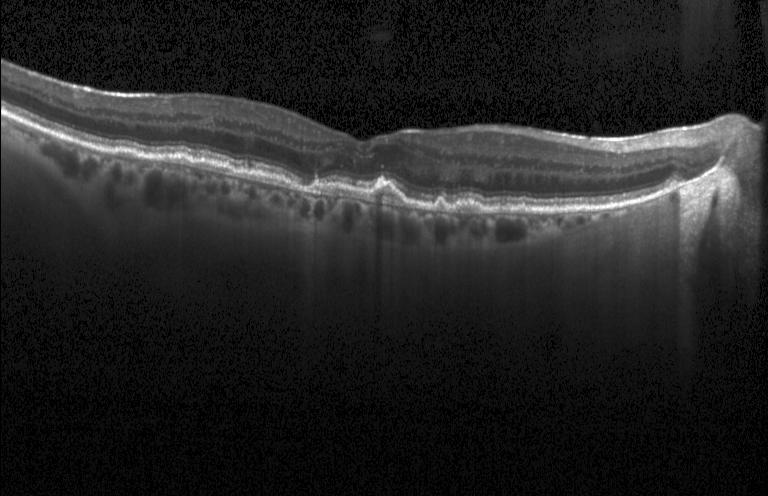 Diagnosis: choroidal neovascularization.